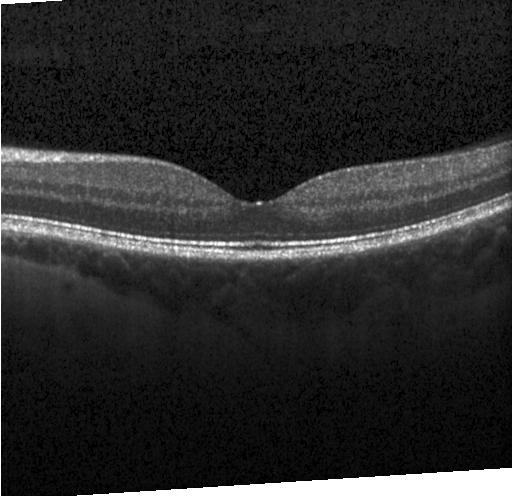 Macular scan, retinal OCT cross-section, instrument: Heidelberg Spectralis — The scan shows neither choroidal neovascularization, diabetic macular edema, nor drusen.